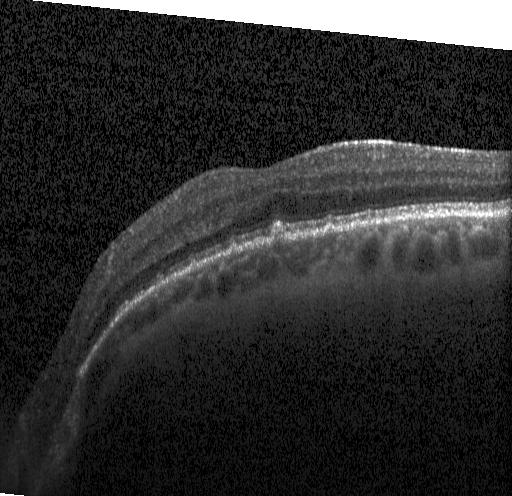
Retinal OCT cross-section — Diagnosis: multiple drusen.